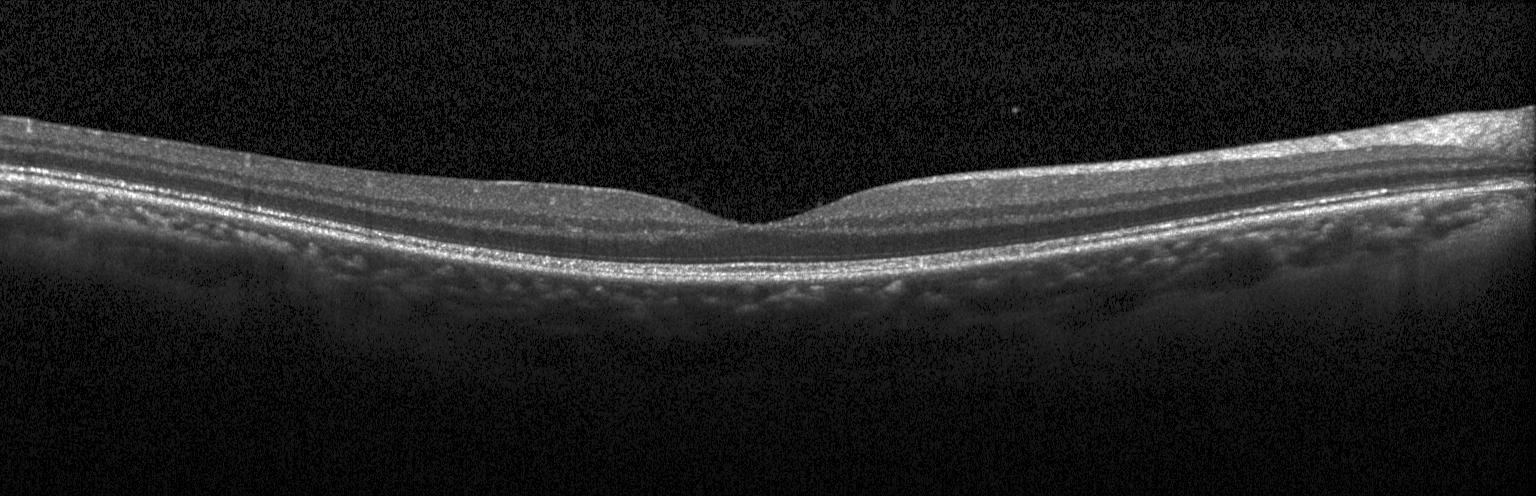

Heidelberg Spectralis OCT system; horizontal scan through the fovea; spectral-domain OCT; retinal OCT cross-section — Macular OCT: no evidence of choroidal neovascularization, diabetic macular edema, or drusen.